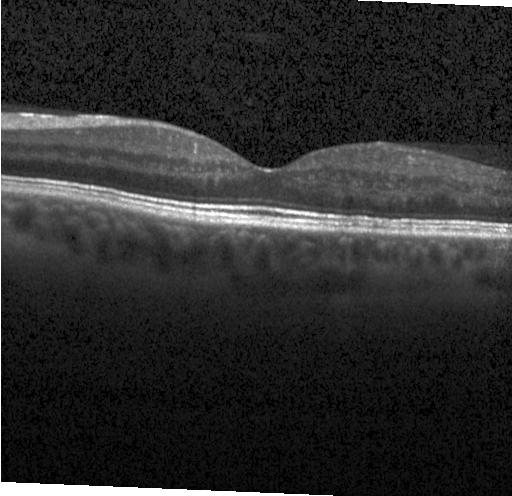

Macular OCT demonstrating no evidence of choroidal neovascularization, diabetic macular edema, or drusen.